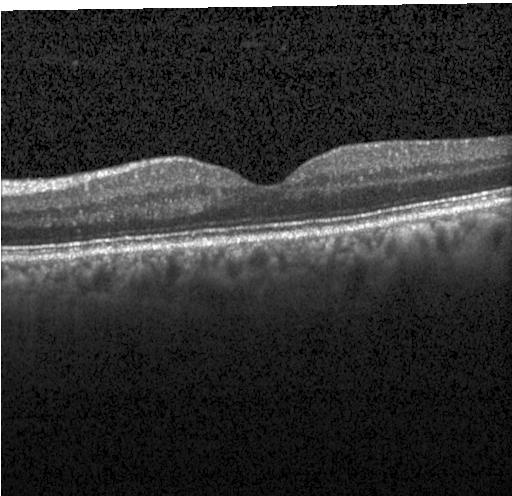

Diagnosis: no choroidal neovascularization, no diabetic macular edema, and no drusen.